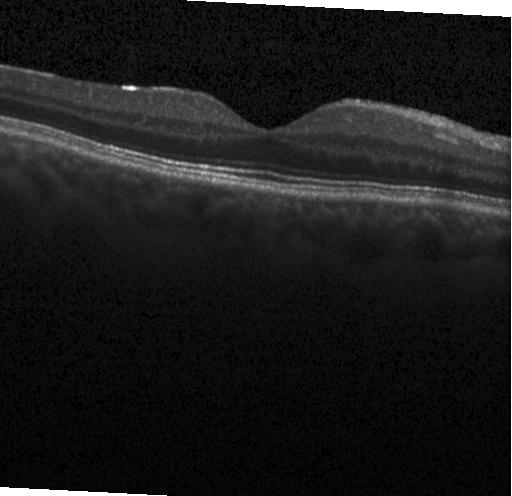

OCT finding: no choroidal neovascularization, no diabetic macular edema, and no drusen.